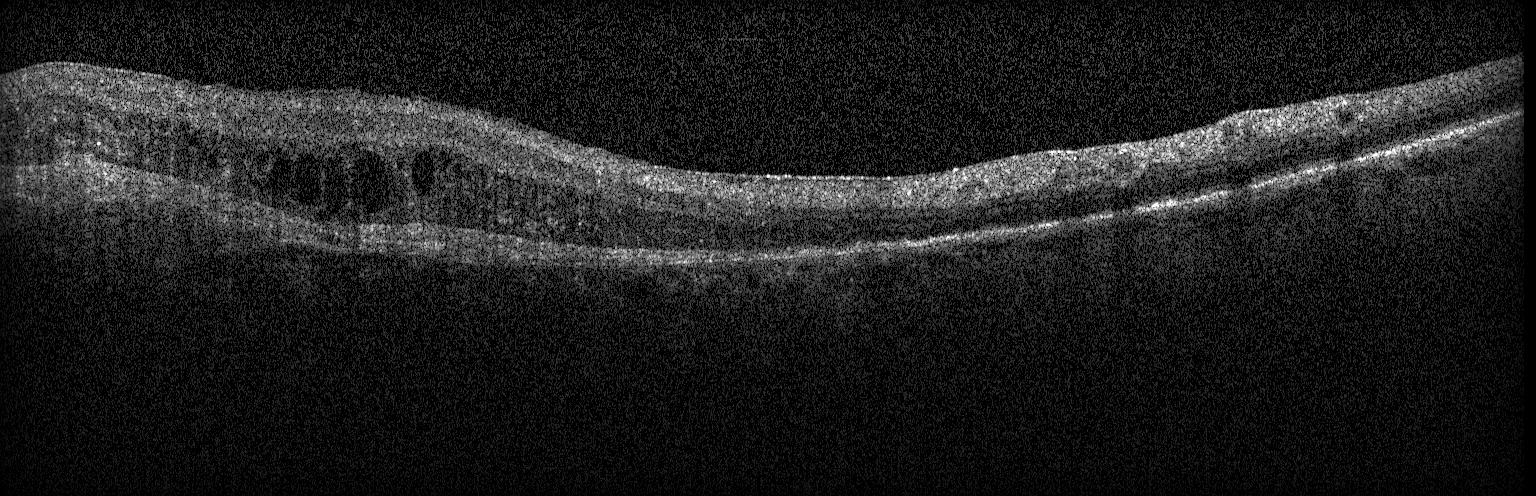 Optical coherence tomography scan · fovea-centered · SD-OCT.
OCT finding: choroidal neovascularization.